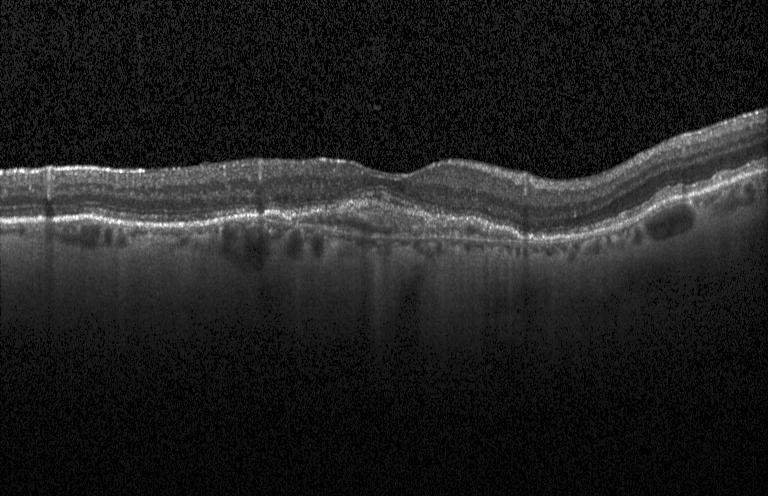 Instrument: Heidelberg Spectralis, OCT B-scan, SD-OCT, horizontal scan through the fovea. Diagnosis: a choroidal neovascular membrane.